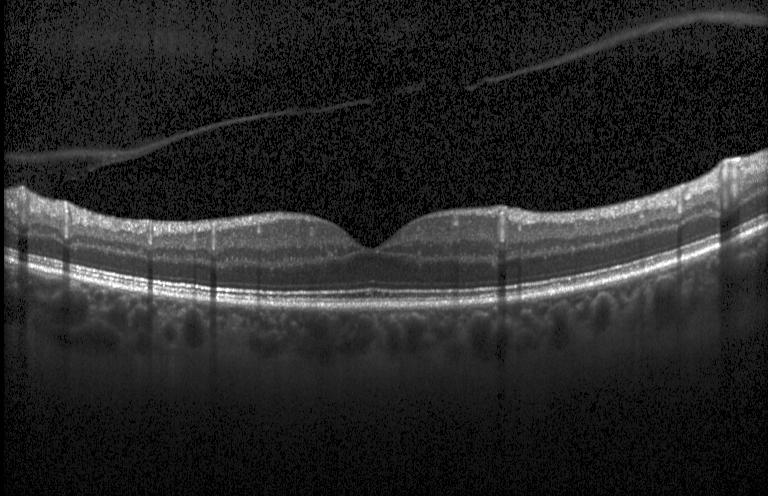
Finding: neither choroidal neovascularization, diabetic macular edema, nor drusen.